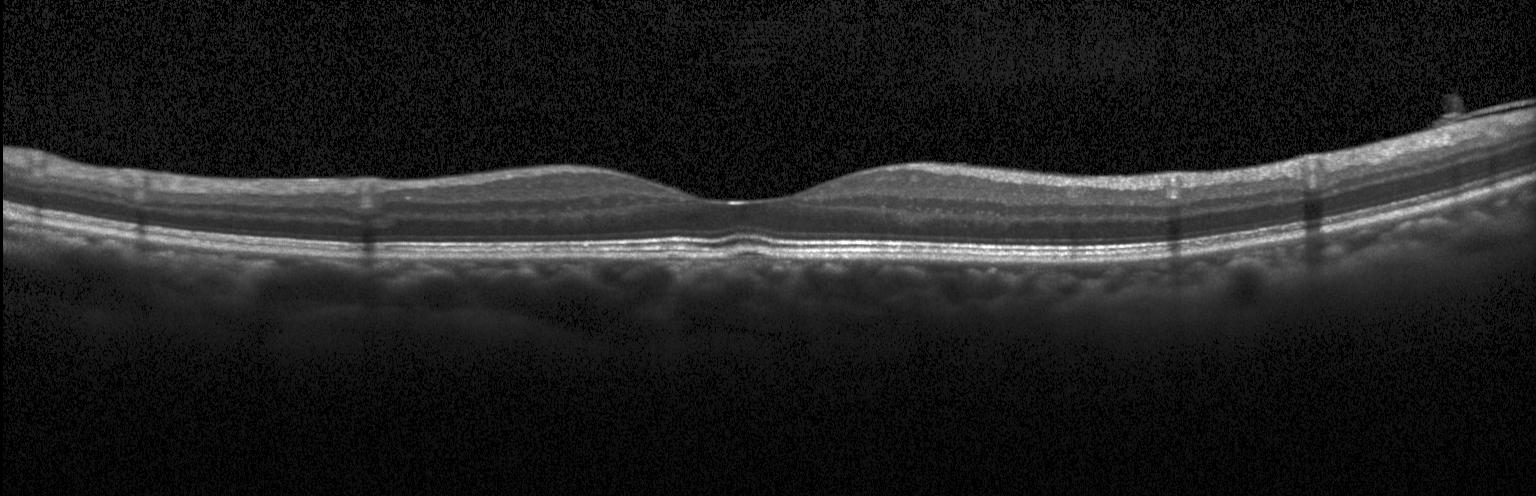
Spectral-domain OCT B-scan: neither choroidal neovascularization, diabetic macular edema, nor drusen.